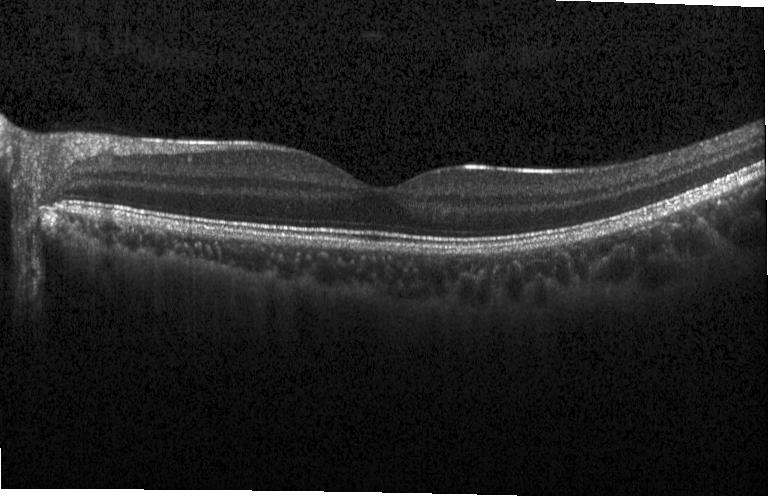 Impression: no choroidal neovascularization, no diabetic macular edema, and no drusen.